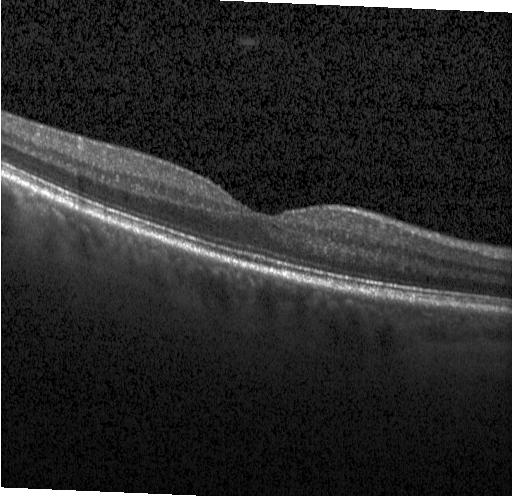
Spectral-domain OCT B-scan: no CNV, DME, or drusen.